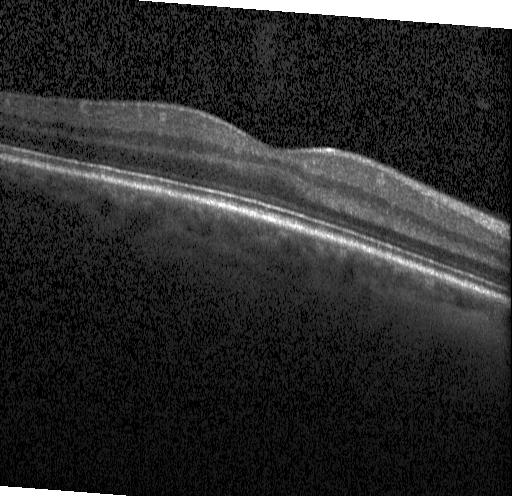 SD-OCT · OCT B-scan.
The scan shows neither CNV, DME, nor drusen.